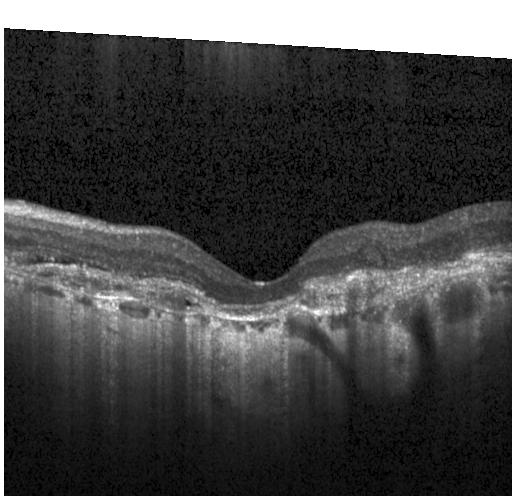
Retinal OCT cross-section. Acquired on a Heidelberg Spectralis
Finding: a choroidal neovascular membrane.